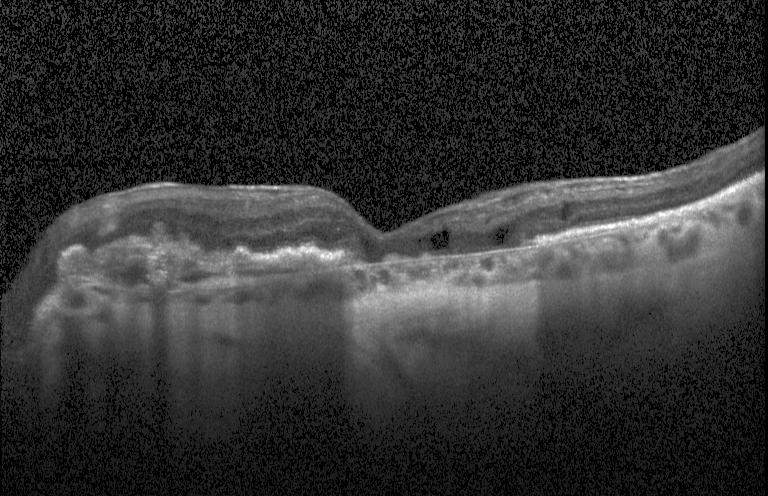 OCT scan showing CNV.